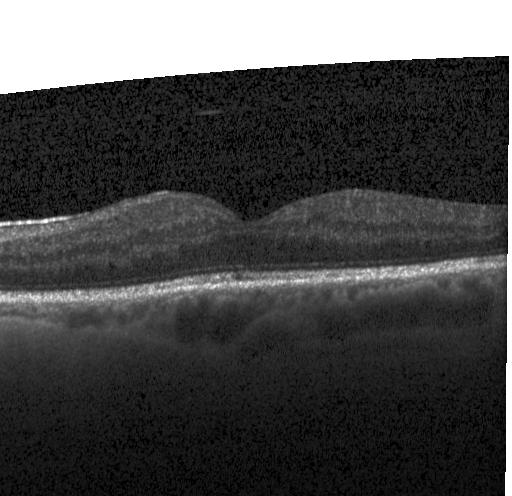

Heidelberg Spectralis; optical coherence tomography scan
Impression: neither choroidal neovascularization, diabetic macular edema, nor drusen.